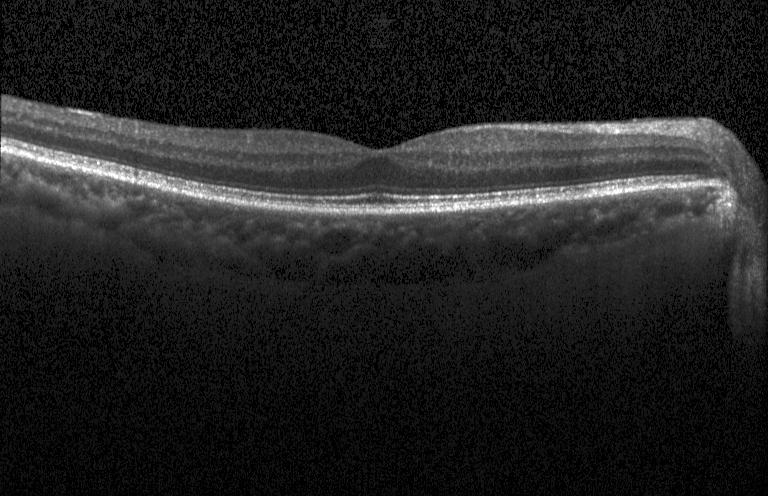 Spectral-domain OCT, fovea-centered, optical coherence tomography scan — Dx: neither choroidal neovascularization, diabetic macular edema, nor drusen.